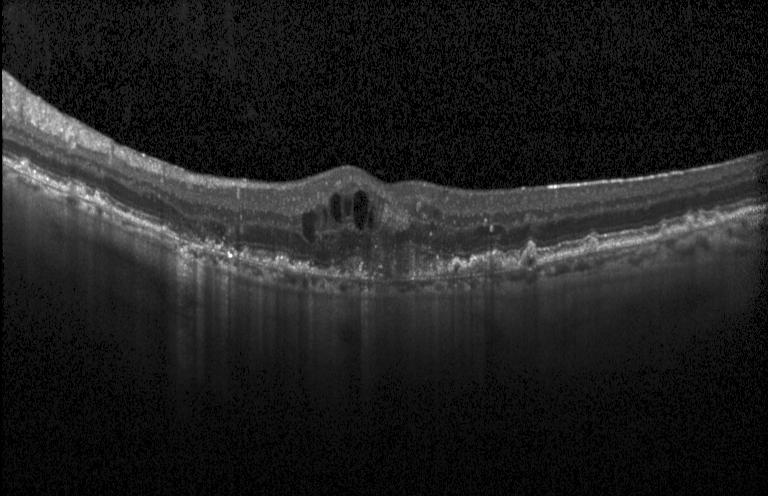 Impression: a choroidal neovascular membrane.